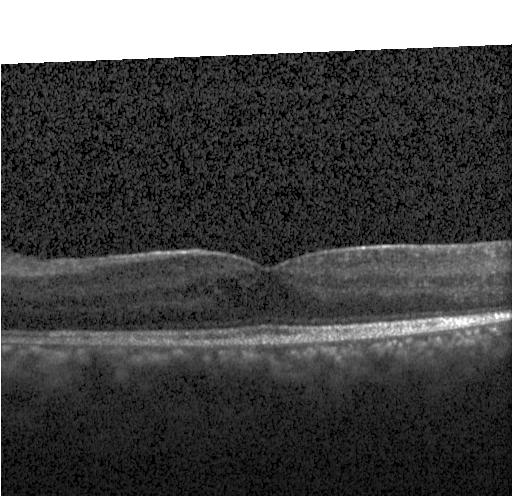 Horizontal scan through the fovea · OCT B-scan — Diabetic macular edema (DME).